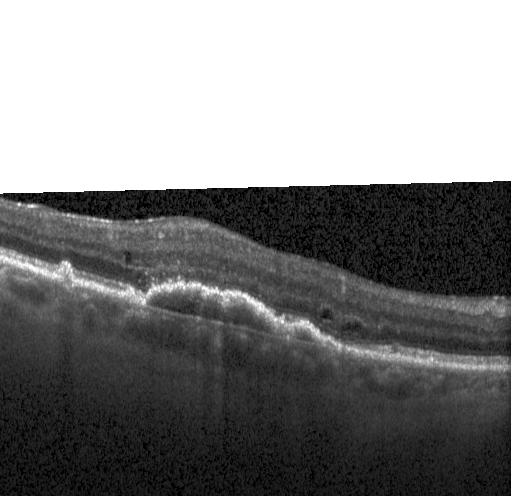
Heidelberg Spectralis; optical coherence tomography scan; through the macula.
A choroidal neovascular membrane.